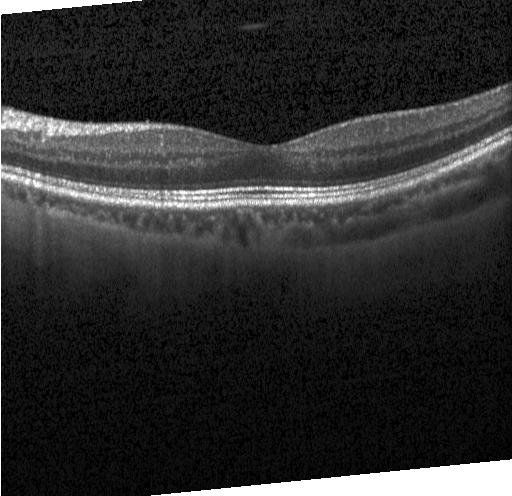 The scan shows no choroidal neovascularization, diabetic macular edema, or drusen.